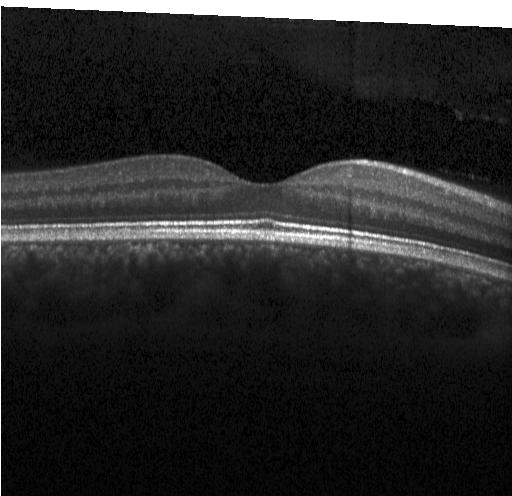 Spectral-domain OCT B-scan: no choroidal neovascularization, no diabetic macular edema, and no drusen.